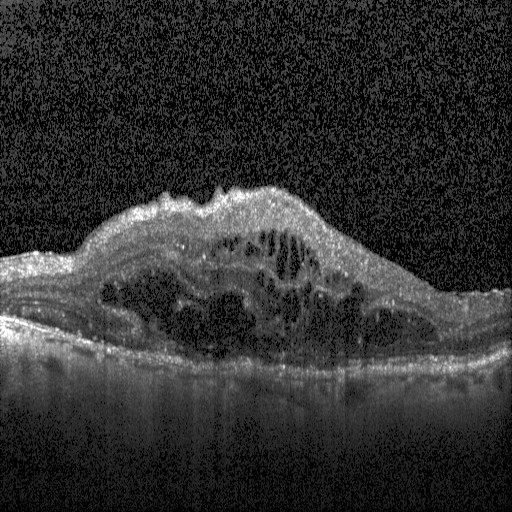

Retinal OCT cross-section. Through the macula.
Diagnosis: diabetic macular edema (DME).